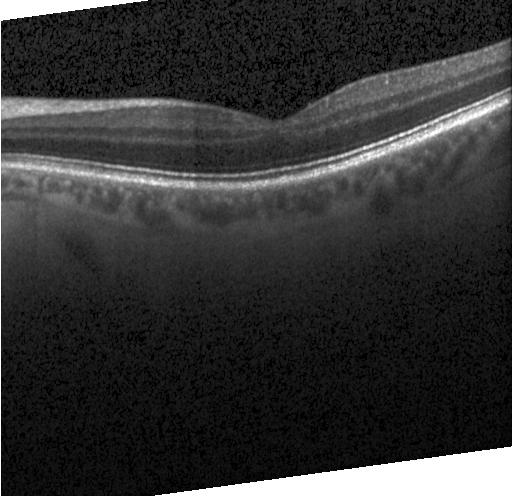 OCT finding: neither choroidal neovascularization, diabetic macular edema, nor drusen.